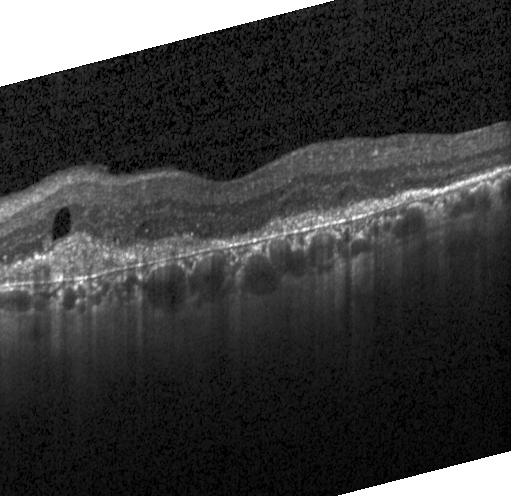

Finding: CNV.